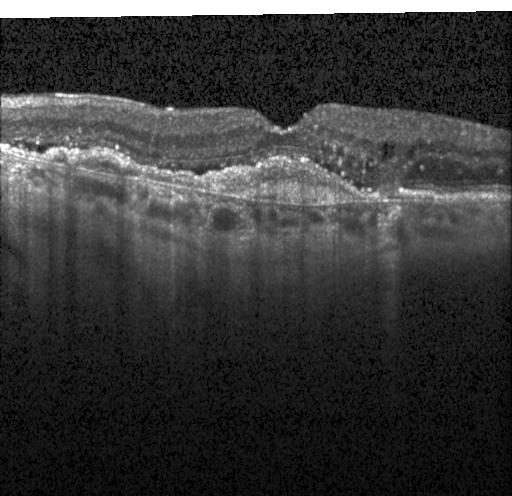
Macular OCT demonstrating a choroidal neovascular membrane.